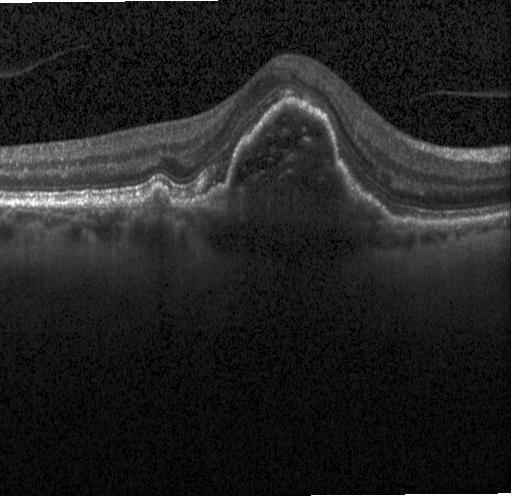

Acquired on a Heidelberg Spectralis. OCT line scan. Spectral-domain OCT. Macular scan
Dx: choroidal neovascularization.